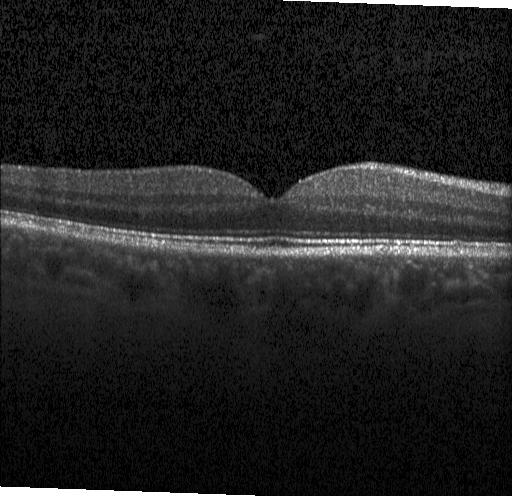

Spectral-domain OCT · fovea-centered · optical coherence tomography scan — OCT finding: neither choroidal neovascularization, diabetic macular edema, nor drusen.